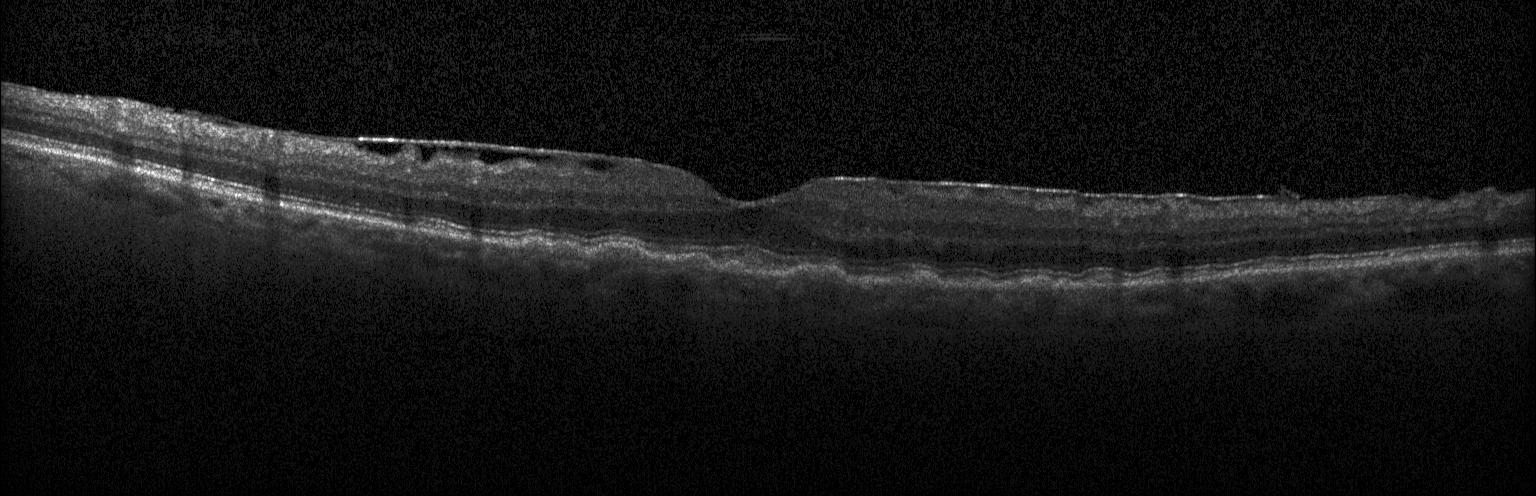

Optical coherence tomography B-scan; spectral-domain optical coherence tomography; instrument: Heidelberg Spectralis; macular scan
Finding: sub-RPE drusenoid deposits.